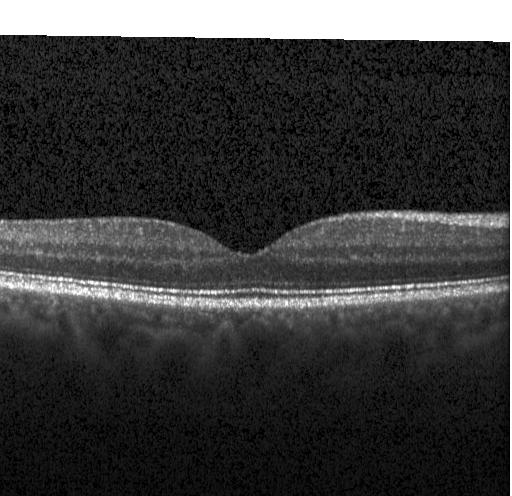
Macular OCT demonstrating no evidence of choroidal neovascularization, diabetic macular edema, or drusen.